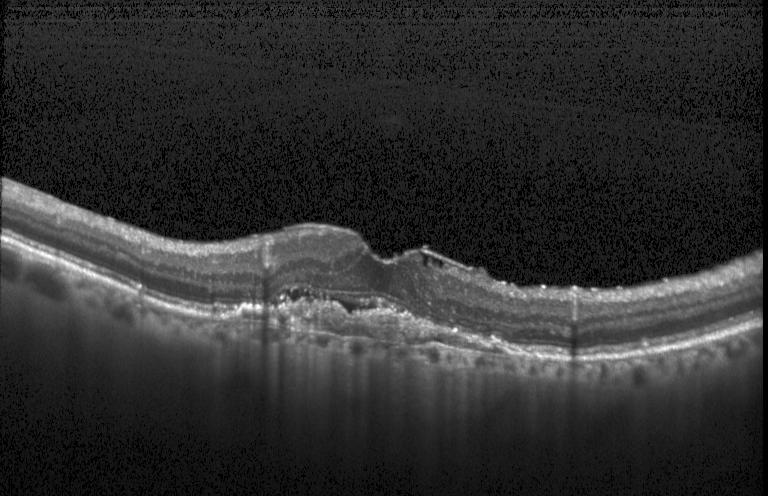 Acquired on a Heidelberg Spectralis. Fovea-centered. Optical coherence tomography B-scan — Assessment: choroidal neovascularization (CNV).